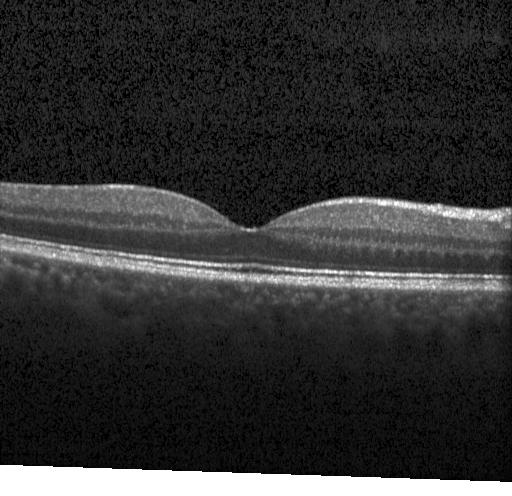
Through the macula. Optical coherence tomography B-scan. SD-OCT. Heidelberg Spectralis.
Diagnosis: neither choroidal neovascularization, diabetic macular edema, nor drusen.